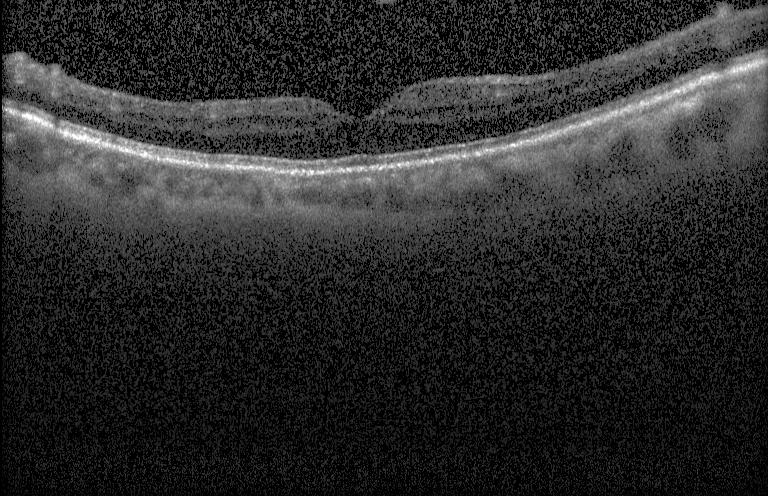 Retinal OCT cross-section showing no choroidal neovascularization, diabetic macular edema, or drusen.